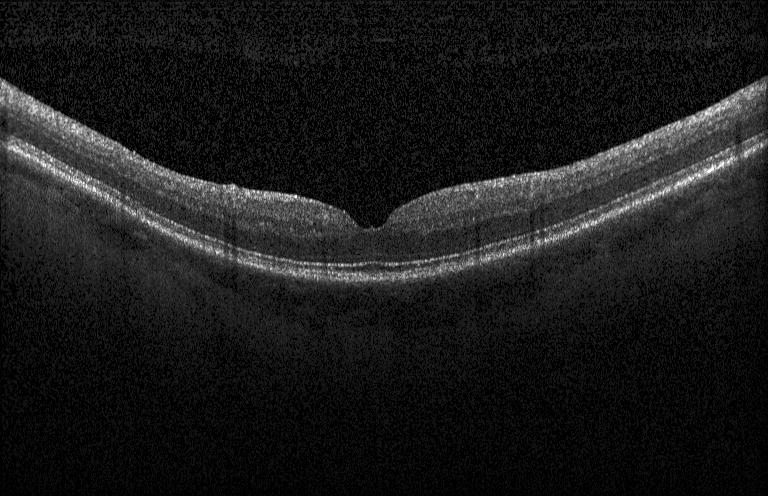 Heidelberg Spectralis, retinal OCT B-scan. Finding: no choroidal neovascularization, diabetic macular edema, or drusen.